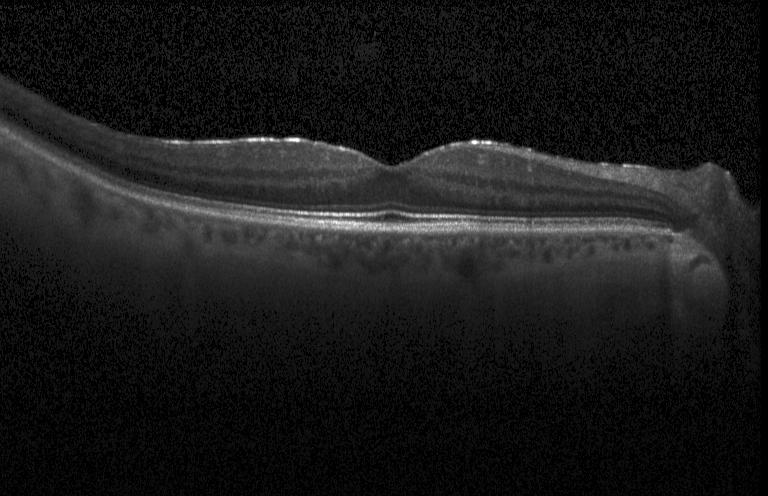 Retinal OCT B-scan · horizontal scan through the fovea.
No choroidal neovascularization, diabetic macular edema, or drusen.